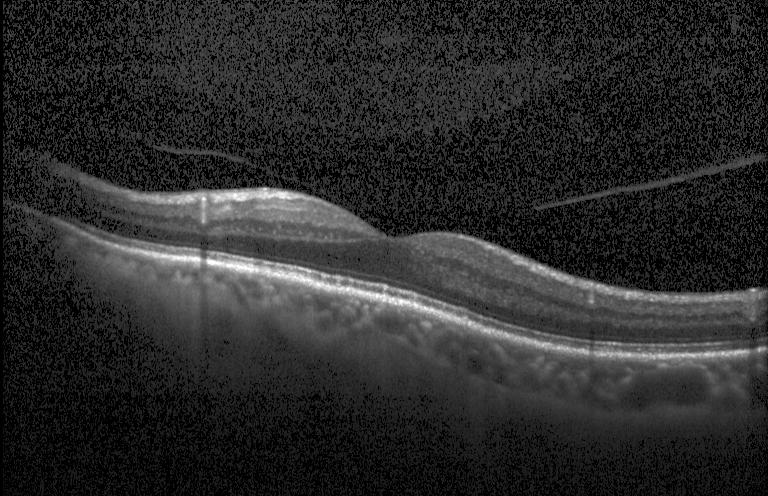 OCT B-scan · SD-OCT · Heidelberg Spectralis · fovea-centered.
Diagnosis: no choroidal neovascularization, no diabetic macular edema, and no drusen.